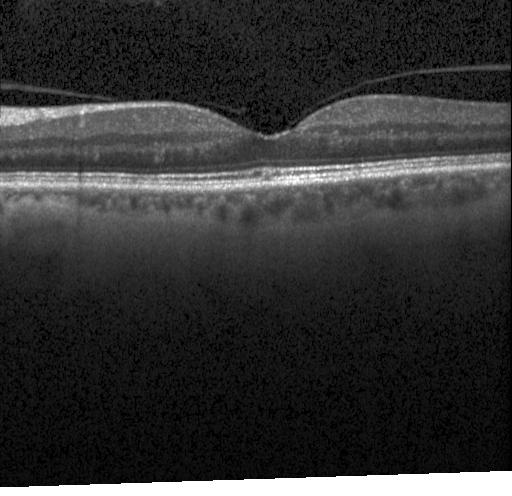 Macular OCT: no evidence of choroidal neovascularization, diabetic macular edema, or drusen.